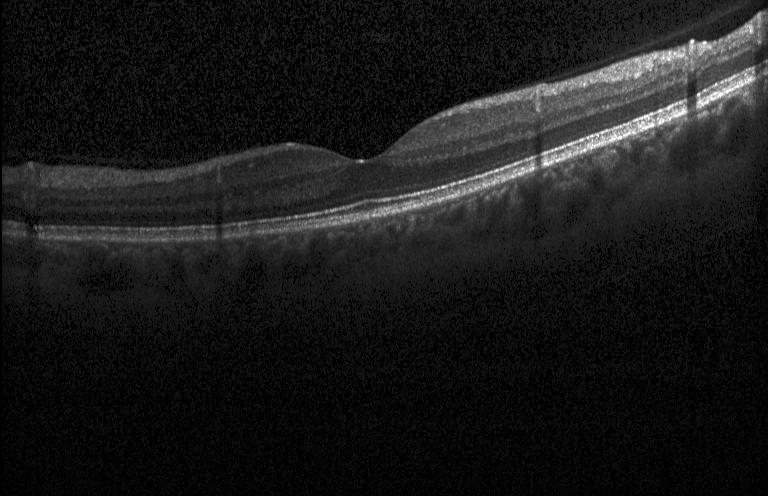

Spectral-domain OCT · instrument: Heidelberg Spectralis · through the macula · retinal OCT cross-section.
OCT finding: no choroidal neovascularization, diabetic macular edema, or drusen.